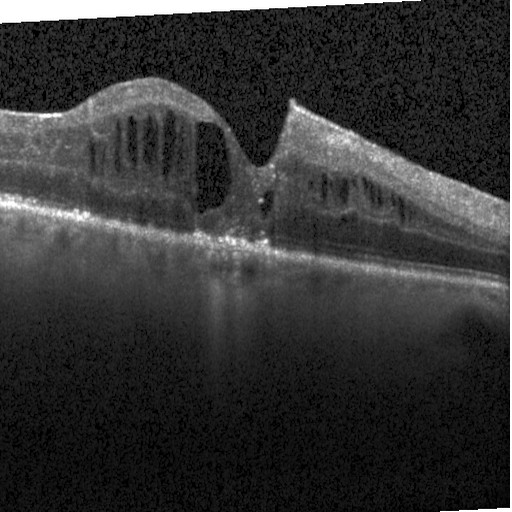 OCT scan showing diabetic macular edema.